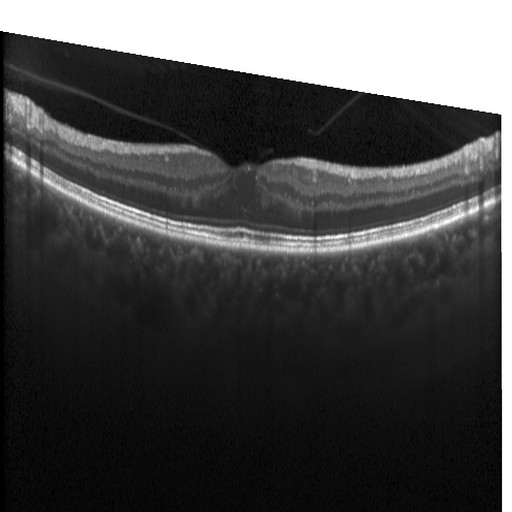
SD-OCT, OCT line scan, Heidelberg Spectralis OCT system, fovea-centered — Diagnosis: diabetic macular edema (DME).